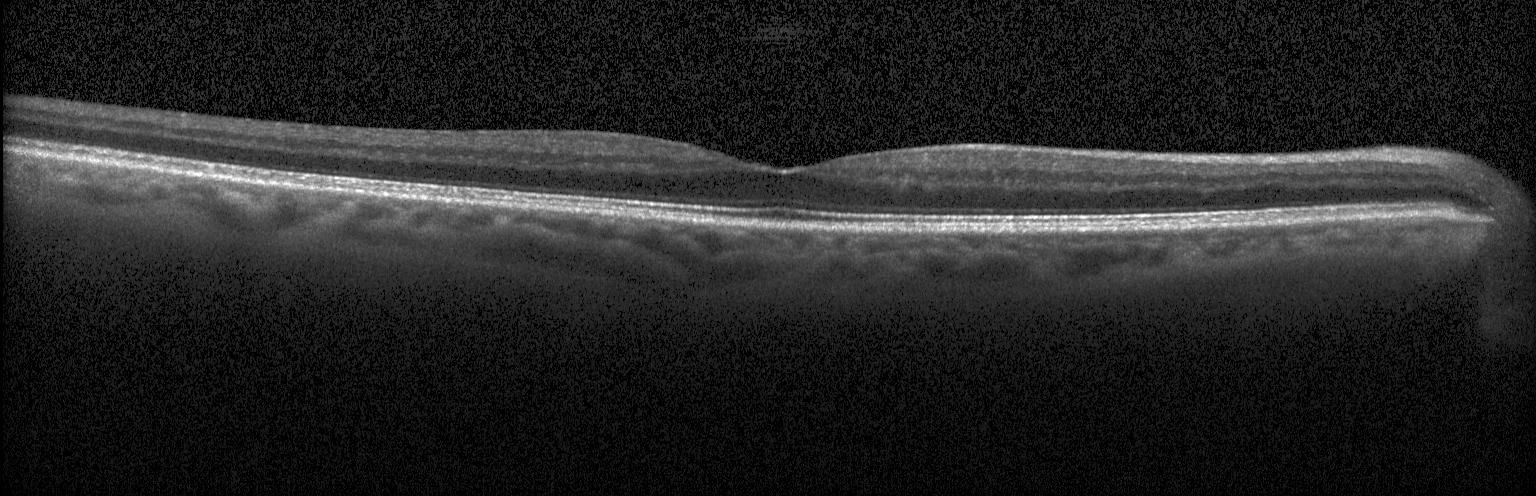

Instrument: Heidelberg Spectralis, OCT B-scan, horizontal scan through the fovea.
Diagnosis: no evidence of choroidal neovascularization, diabetic macular edema, or drusen.